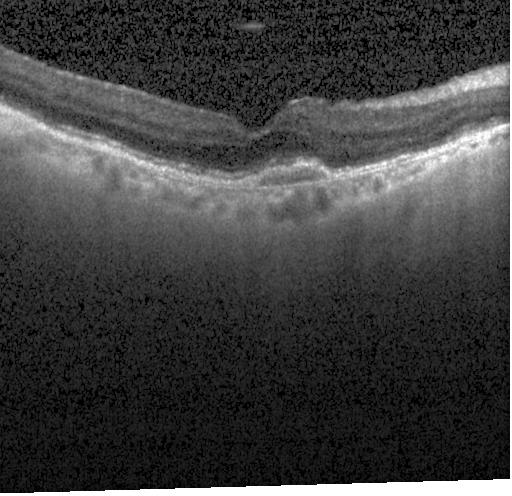
A choroidal neovascular membrane.